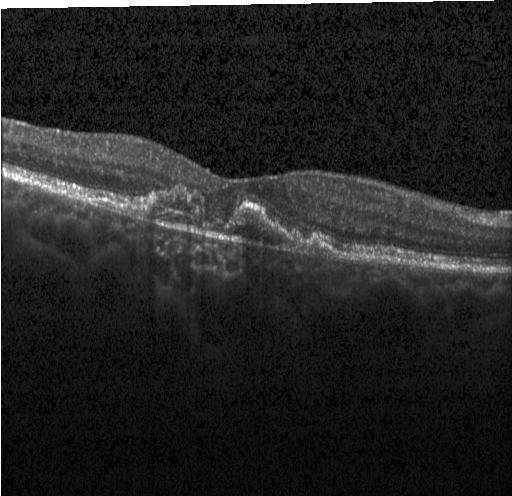 OCT scan showing choroidal neovascularization (CNV).